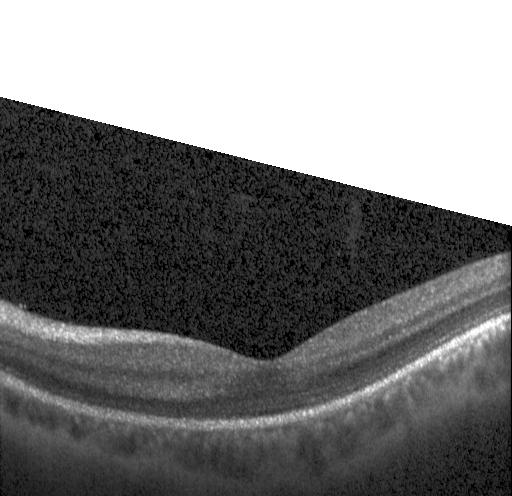
Impression: no choroidal neovascularization, diabetic macular edema, or drusen.